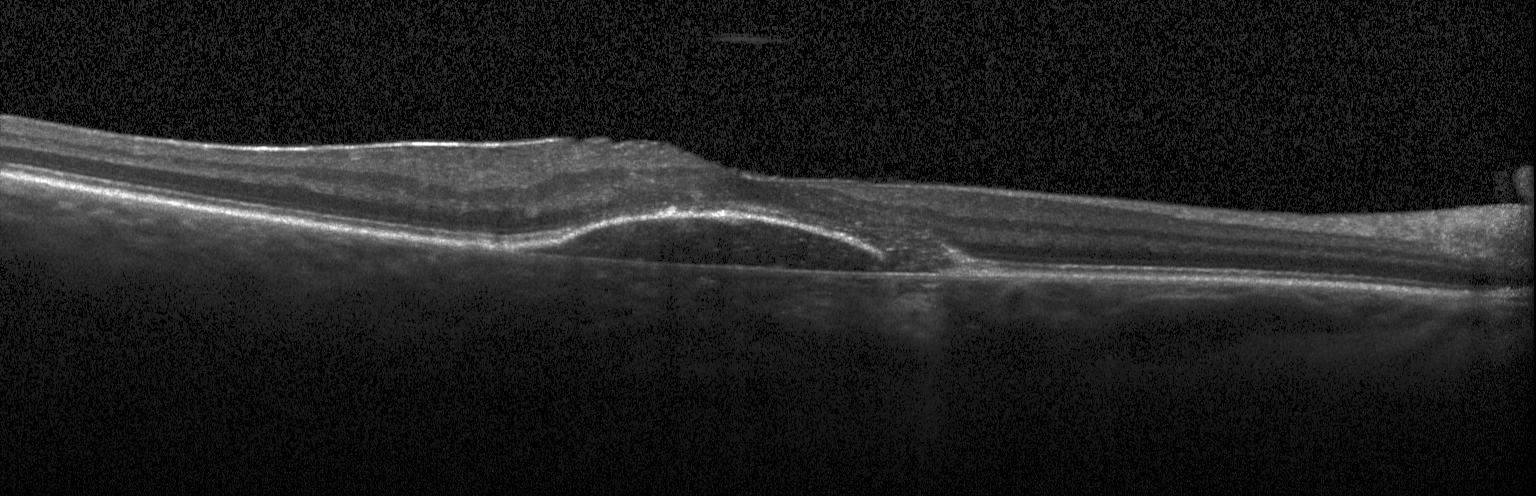

Optical coherence tomography B-scan
This B-scan demonstrates choroidal neovascularization (CNV).